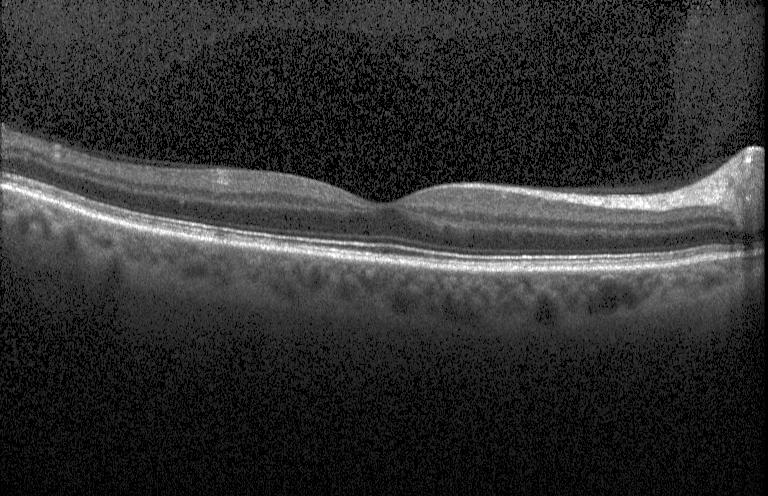 Through the macula; retinal OCT B-scan. Macular OCT: no CNV, DME, or drusen.